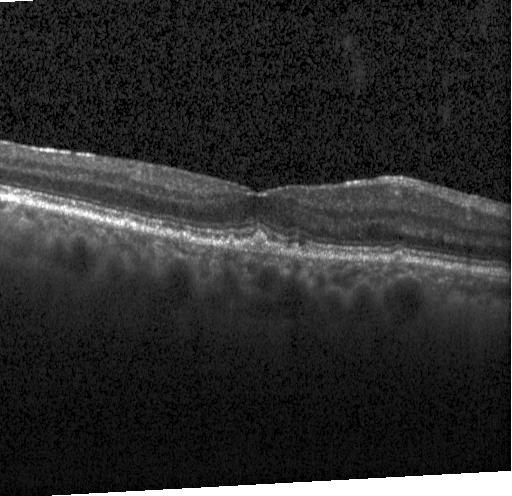 Horizontal scan through the fovea. Spectral-domain OCT. OCT line scan. The scan shows drusen.